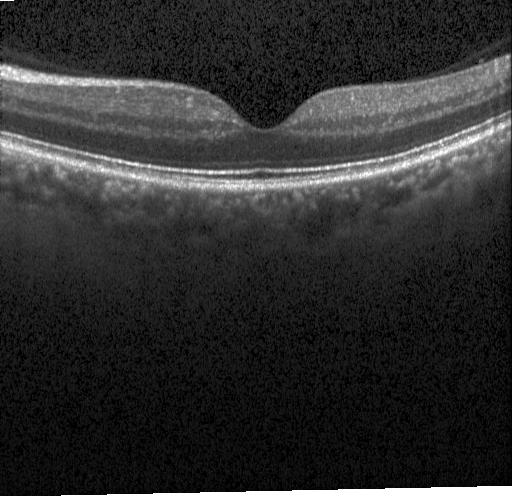
OCT B-scan, Heidelberg Spectralis OCT system. Finding: no evidence of CNV, DME, or drusen.